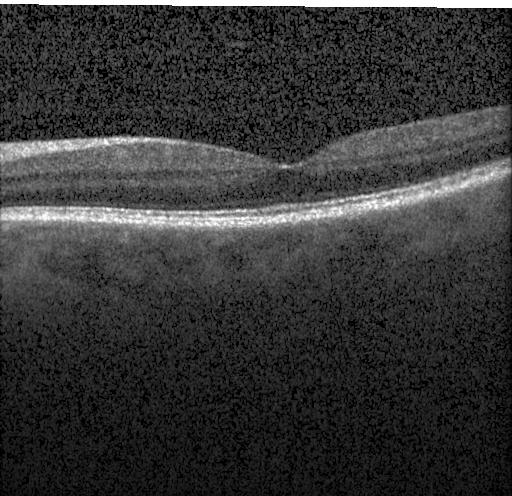

Neither CNV, DME, nor drusen.